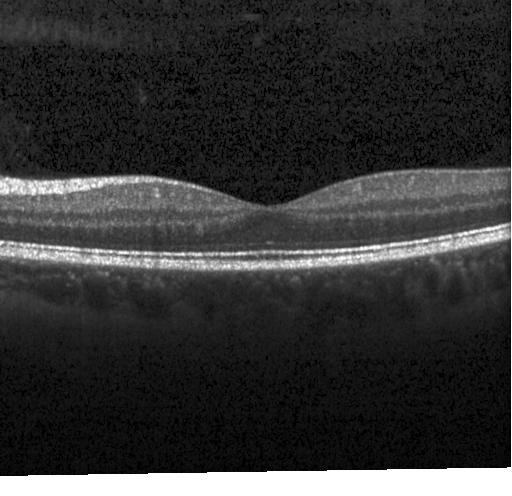
Retinal OCT cross-section
Finding: no CNV, DME, or drusen.